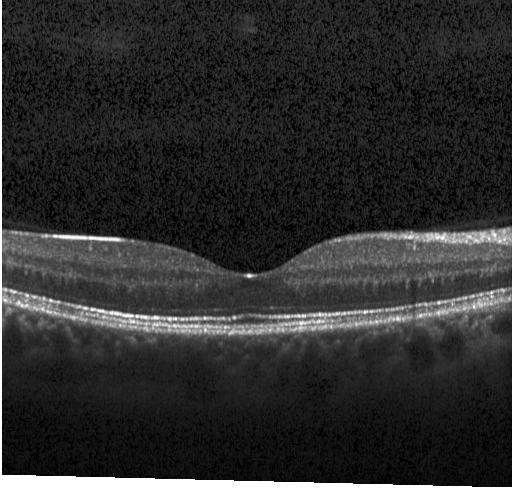

Instrument: Heidelberg Spectralis · optical coherence tomography B-scan.
Diagnosis: no CNV, no DME, and no drusen.